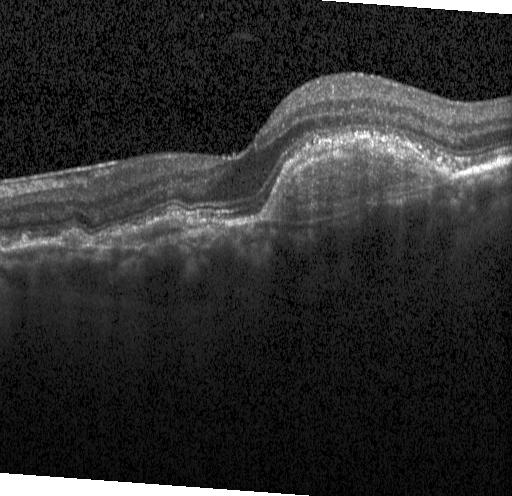

Retinal OCT B-scan. Macular OCT: choroidal neovascularization (CNV).